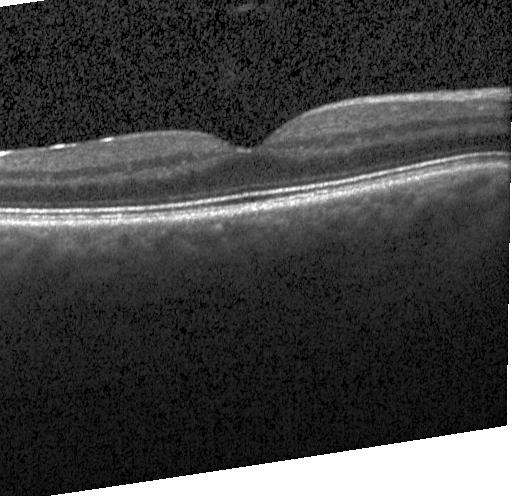 Impression: no choroidal neovascularization, diabetic macular edema, or drusen.